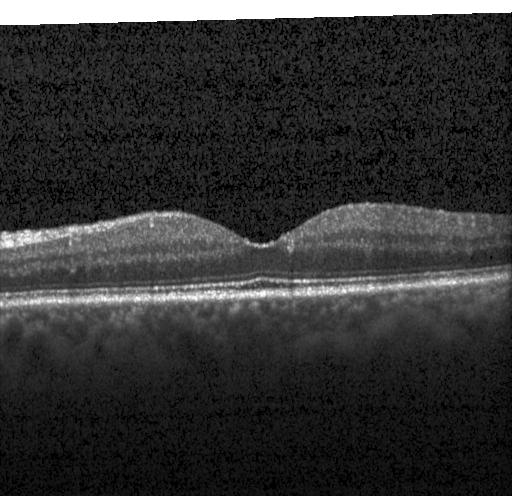 Heidelberg Spectralis OCT system; centered on the fovea; retinal OCT B-scan — Finding: no CNV, DME, or drusen.